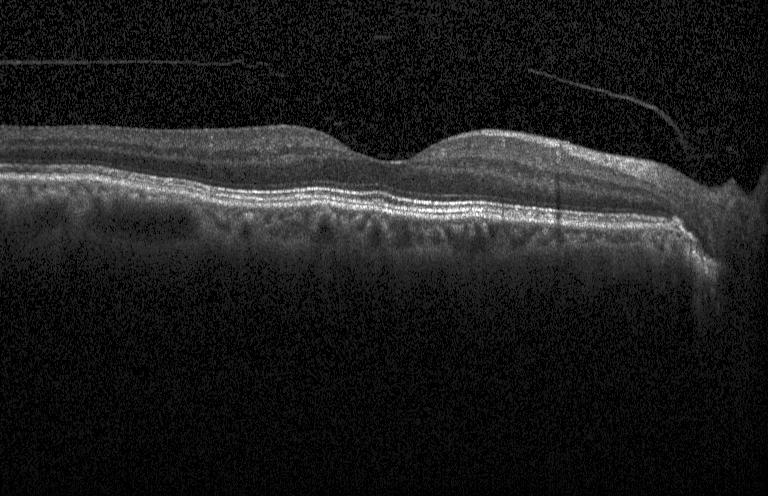
Optical coherence tomography scan — Finding: no evidence of choroidal neovascularization, diabetic macular edema, or drusen.